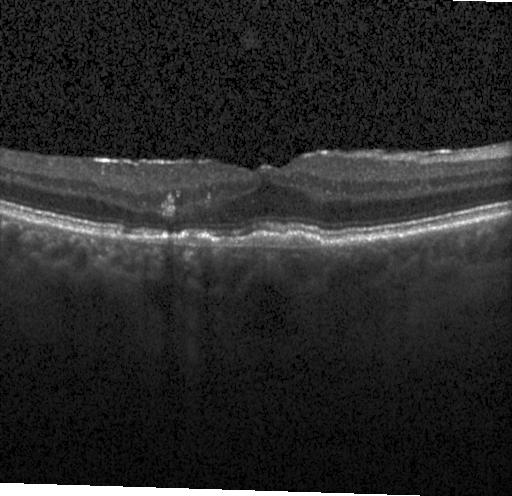

Retinal OCT B-scan; horizontal scan through the fovea
Choroidal neovascularization.